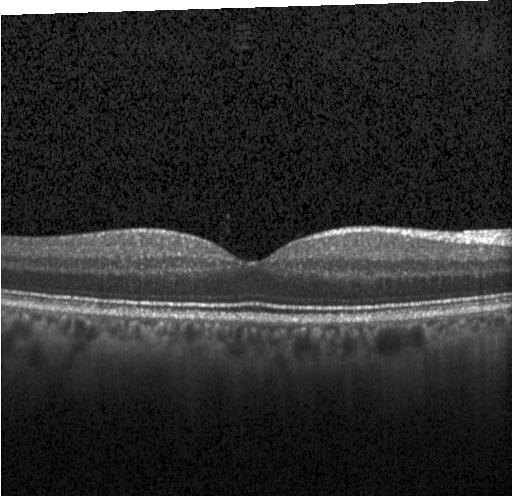

Through the macula. OCT B-scan. Instrument: Heidelberg Spectralis. Spectral-domain optical coherence tomography.
No choroidal neovascularization, no diabetic macular edema, and no drusen.